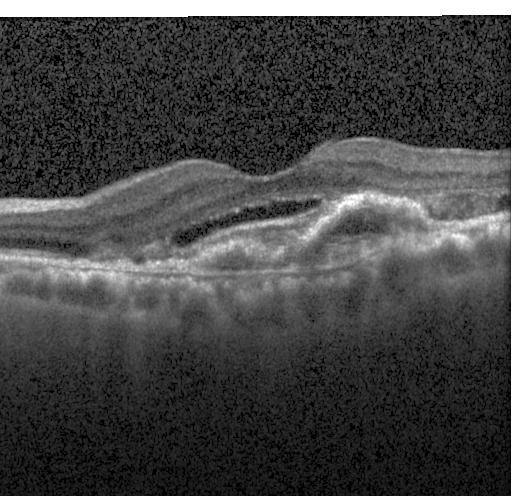
Assessment: a choroidal neovascular membrane.